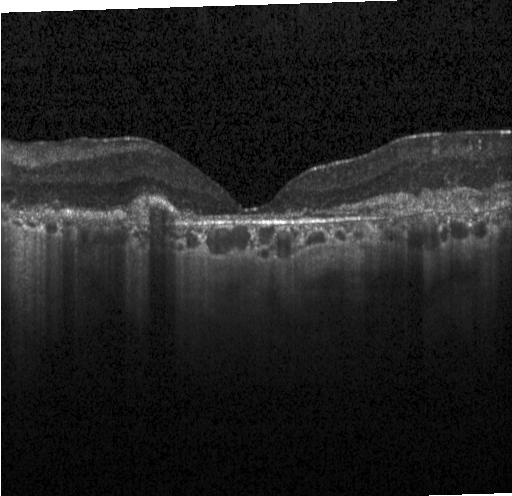
Spectral-domain optical coherence tomography, acquired on a Heidelberg Spectralis, fovea-centered, OCT line scan.
Assessment: a choroidal neovascular membrane.